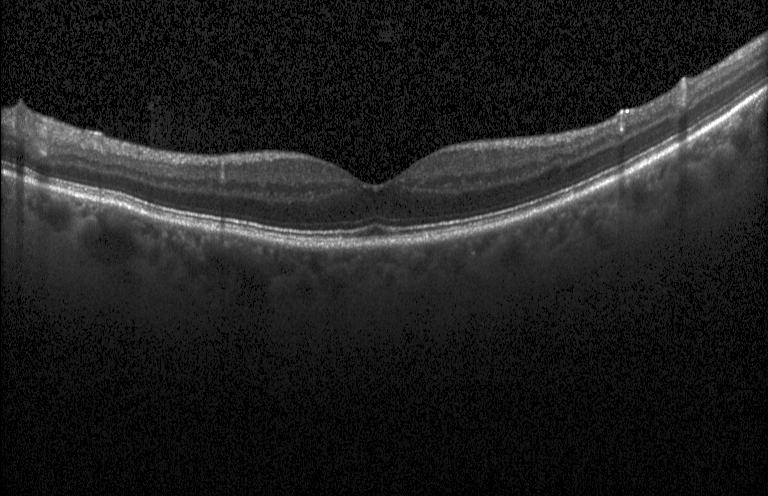
Retinal OCT B-scan.
No evidence of choroidal neovascularization, diabetic macular edema, or drusen.